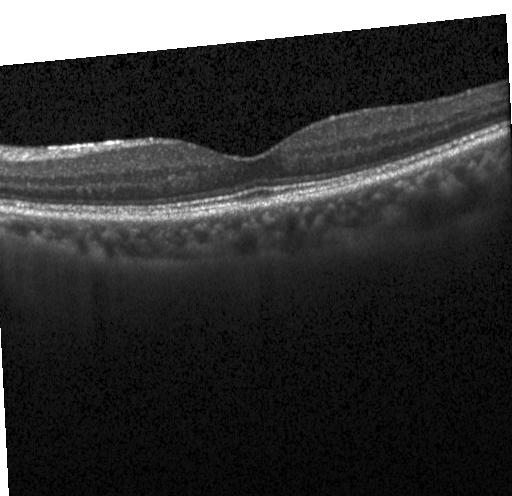
The scan shows no choroidal neovascularization, diabetic macular edema, or drusen.